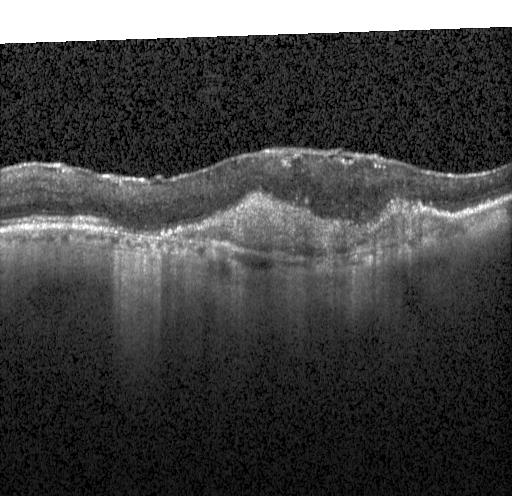

Dx: CNV.